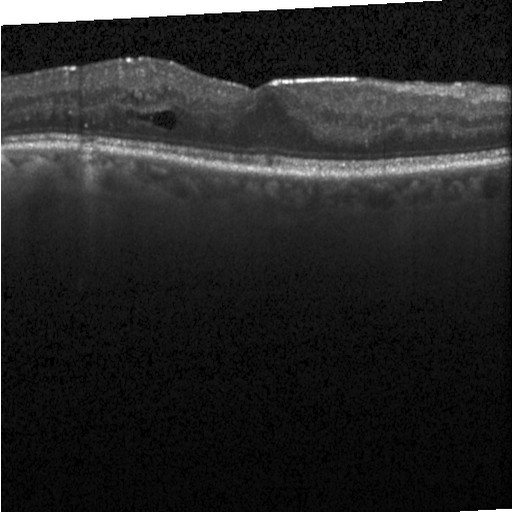
Heidelberg Spectralis OCT system, OCT line scan — Dx: diabetic macular edema.